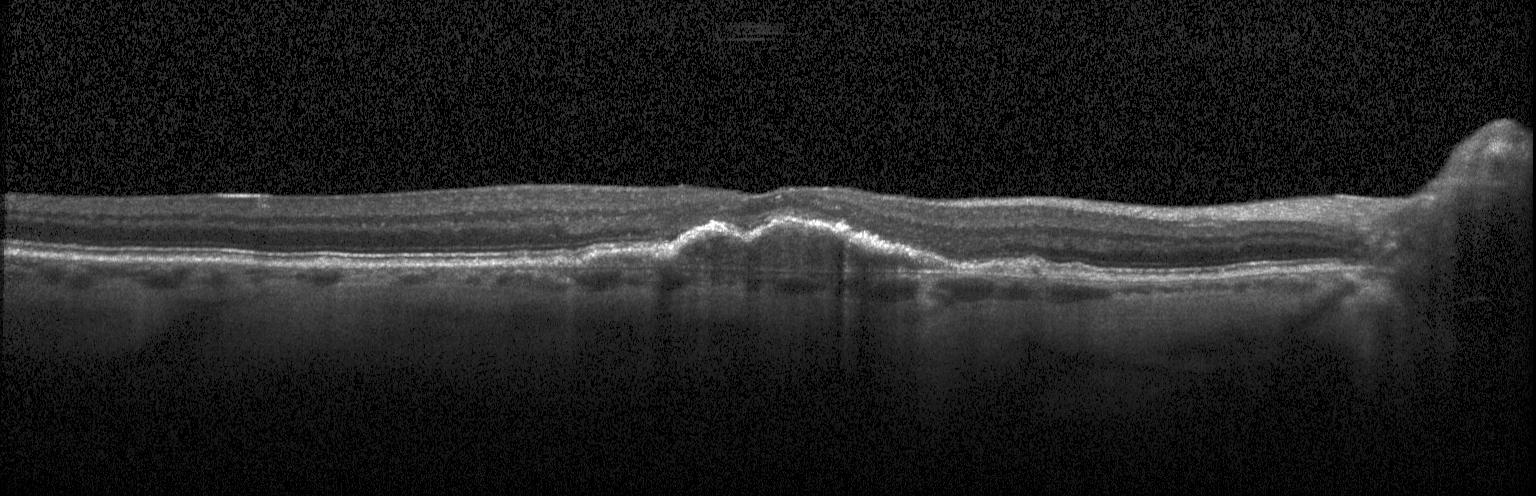 OCT B-scan.
A choroidal neovascular membrane.